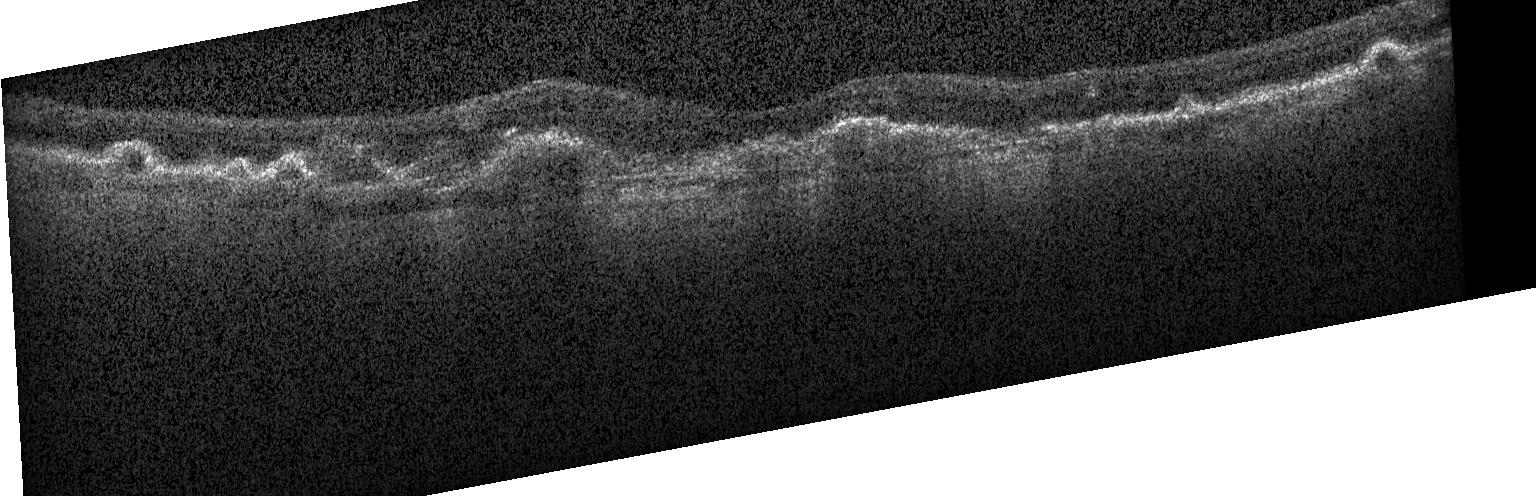 Optical coherence tomography scan · spectral-domain optical coherence tomography
CNV.